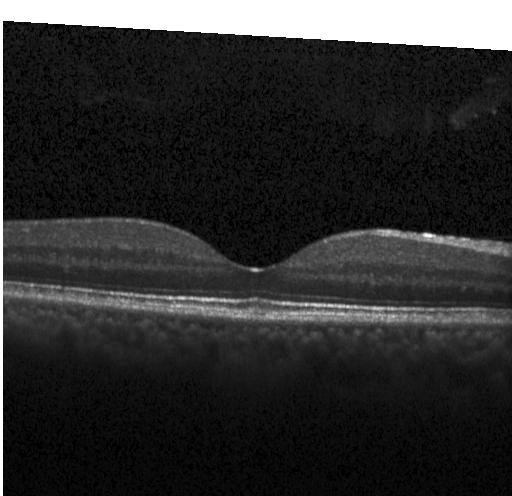 This B-scan demonstrates no choroidal neovascularization, no diabetic macular edema, and no drusen.